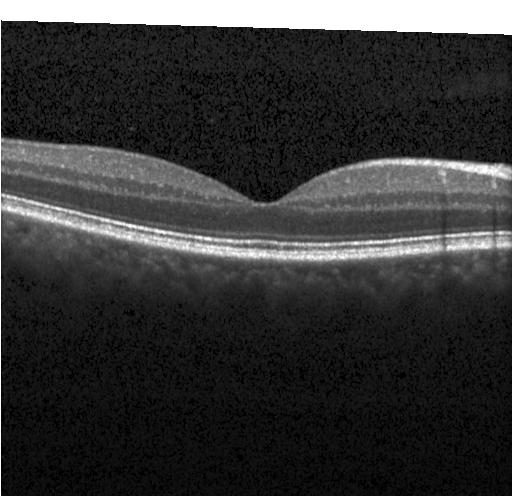
Impression: neither choroidal neovascularization, diabetic macular edema, nor drusen.